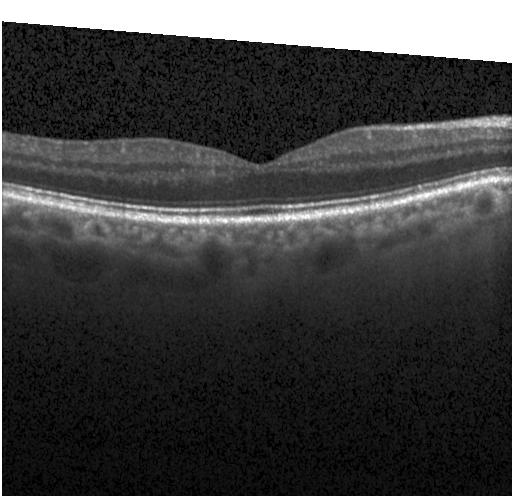 Retinal OCT cross-section showing no evidence of choroidal neovascularization, diabetic macular edema, or drusen.